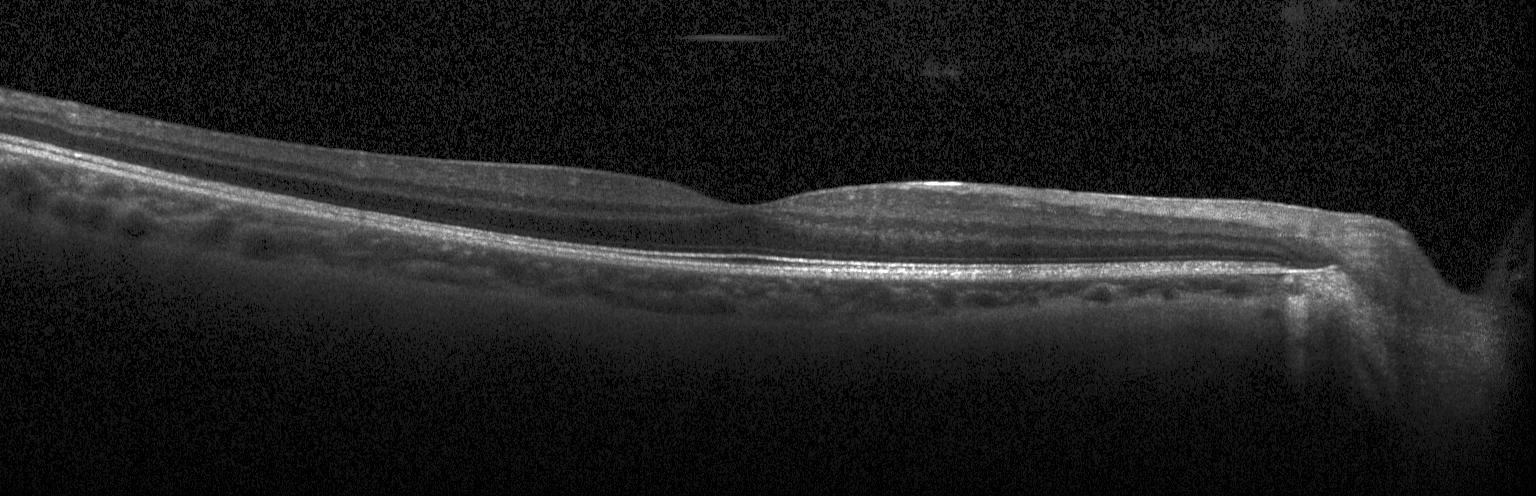

Optical coherence tomography scan — Impression: no choroidal neovascularization, no diabetic macular edema, and no drusen.